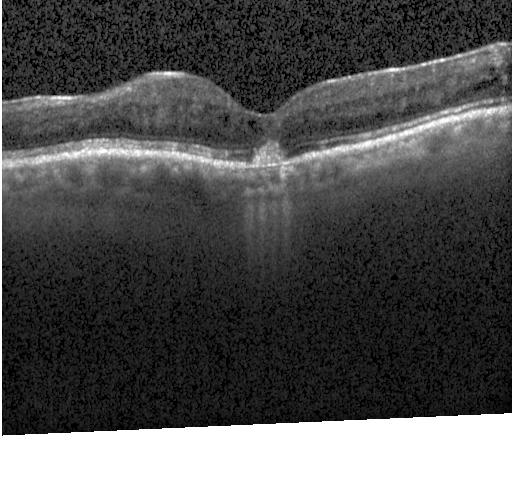 Finding: choroidal neovascularization.